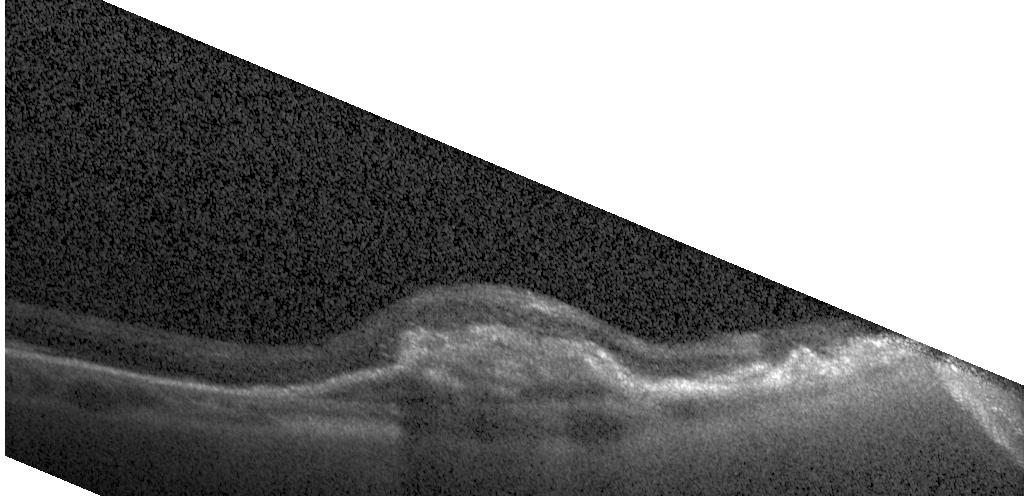 Horizontal scan through the fovea; OCT line scan; SD-OCT — Impression: a choroidal neovascular membrane.